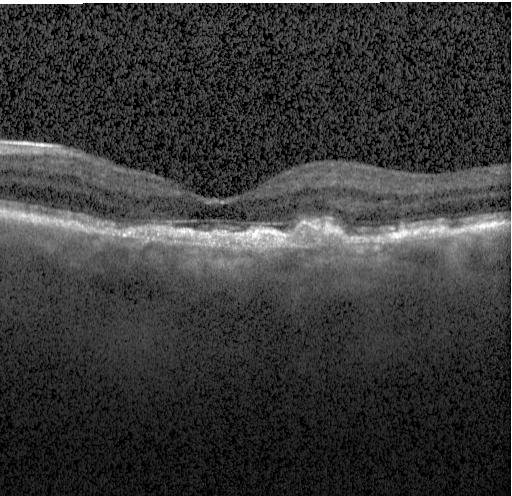 Macular OCT demonstrating a choroidal neovascular membrane.